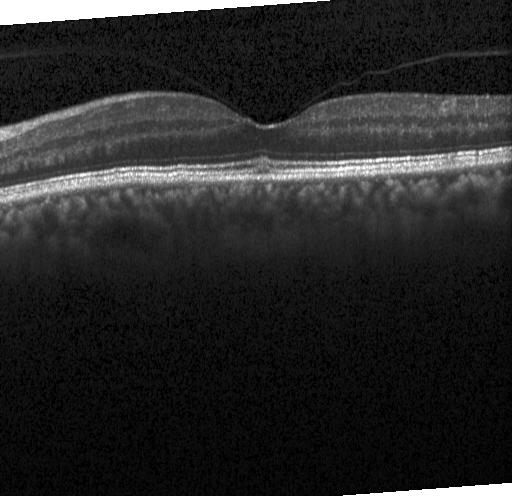
OCT finding: no CNV, DME, or drusen.